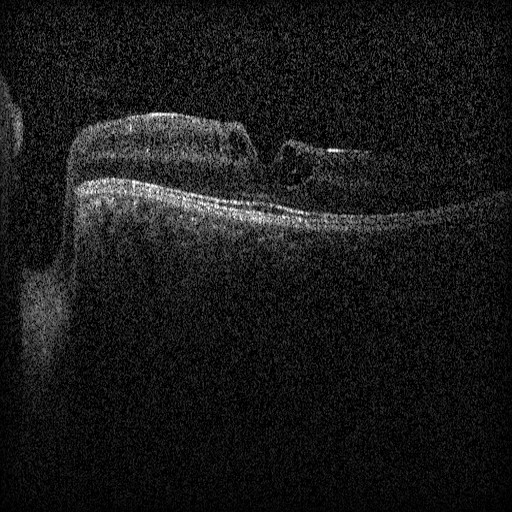 Optical coherence tomography scan. OCT finding: DME.